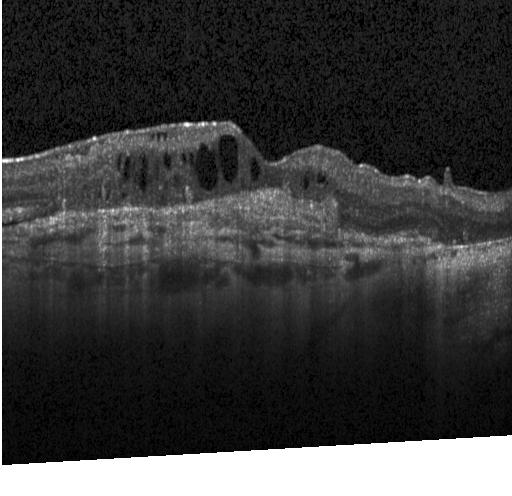

OCT scan showing a choroidal neovascular membrane.